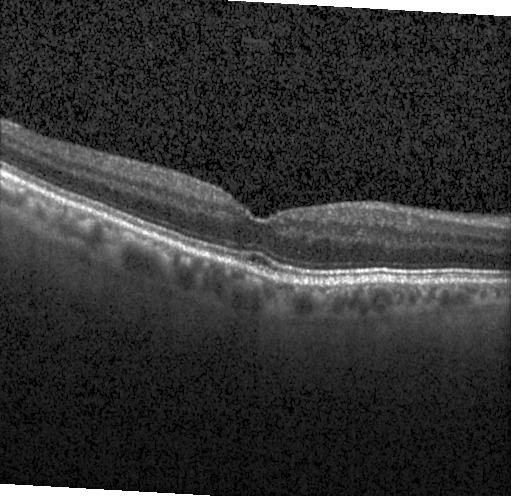

Impression: no choroidal neovascularization, diabetic macular edema, or drusen.